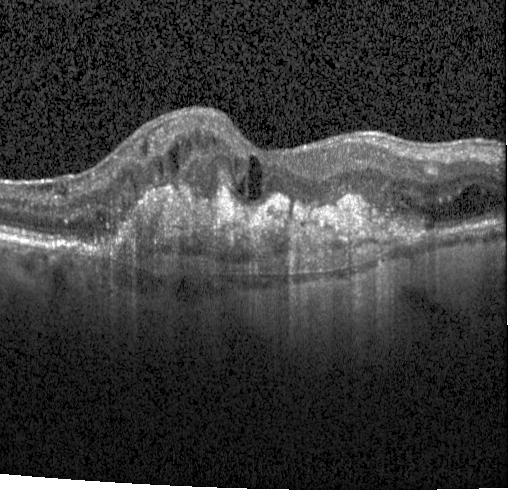

Retinal OCT B-scan · instrument: Heidelberg Spectralis. Dx: a choroidal neovascular membrane.